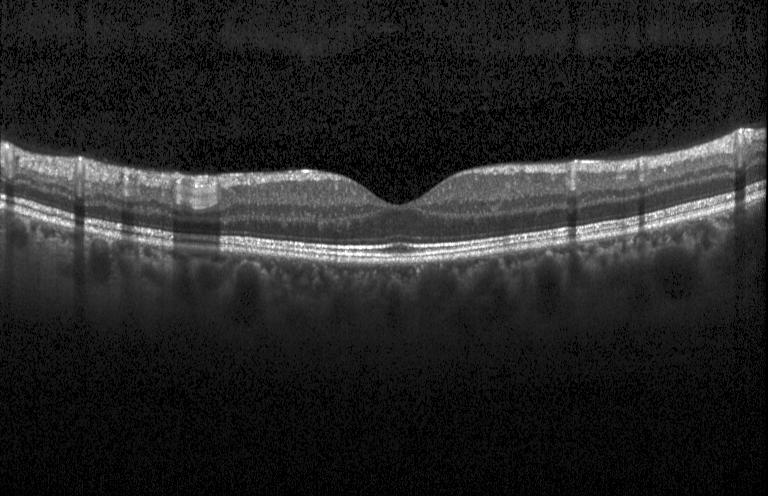
Acquired on a Heidelberg Spectralis · OCT B-scan — The scan shows neither CNV, DME, nor drusen.